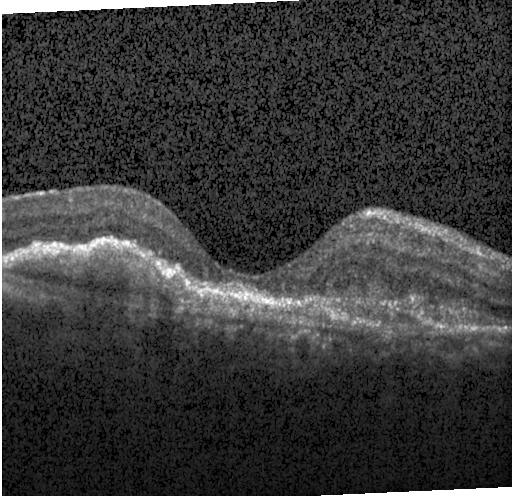
Heidelberg Spectralis · spectral-domain optical coherence tomography · macular scan · optical coherence tomography B-scan.
Finding: a choroidal neovascular membrane.